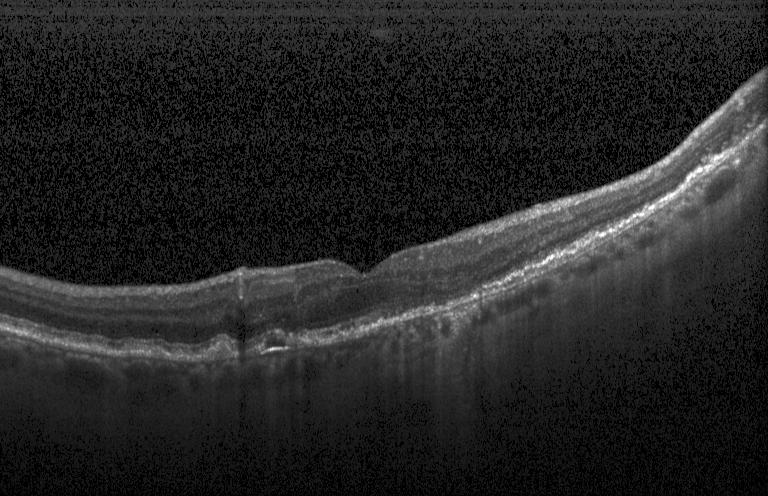 OCT line scan; Heidelberg Spectralis OCT system
Finding: a choroidal neovascular membrane.